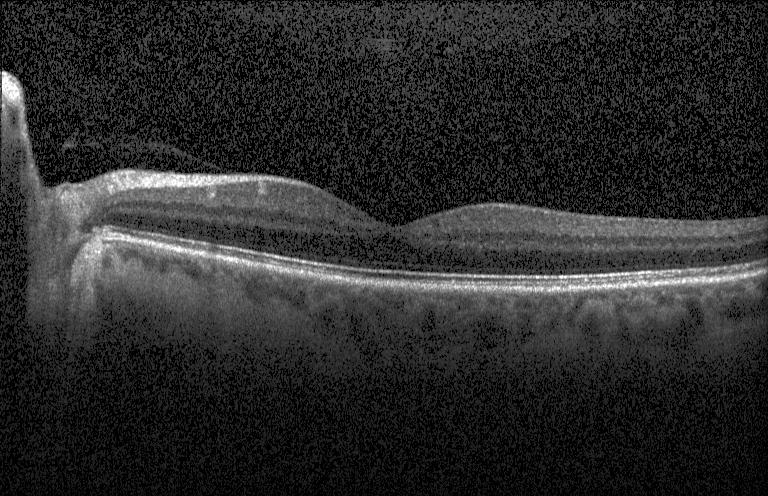 OCT B-scan; Heidelberg Spectralis
OCT finding: no evidence of CNV, DME, or drusen.